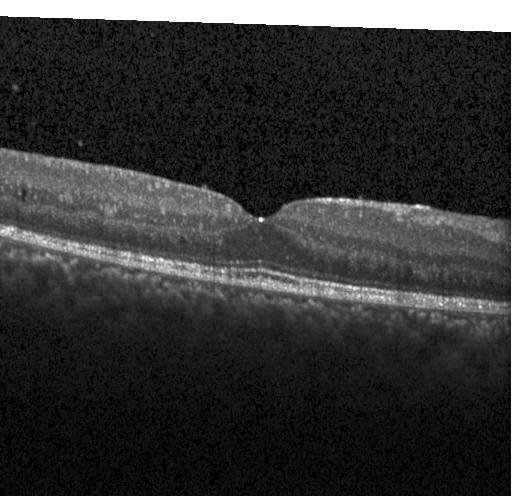 Heidelberg Spectralis, retinal OCT cross-section, fovea-centered, spectral-domain optical coherence tomography. Dx: diabetic macular edema (DME).